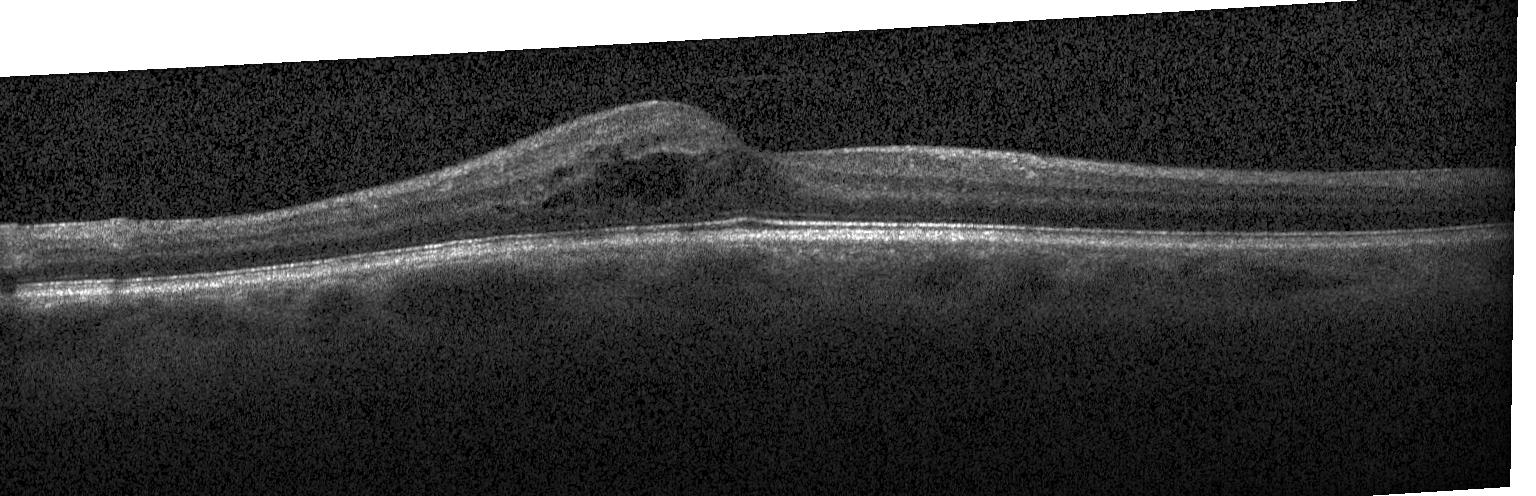 Optical coherence tomography B-scan · through the macula · instrument: Heidelberg Spectralis · SD-OCT.
OCT finding: diabetic macular edema (DME).